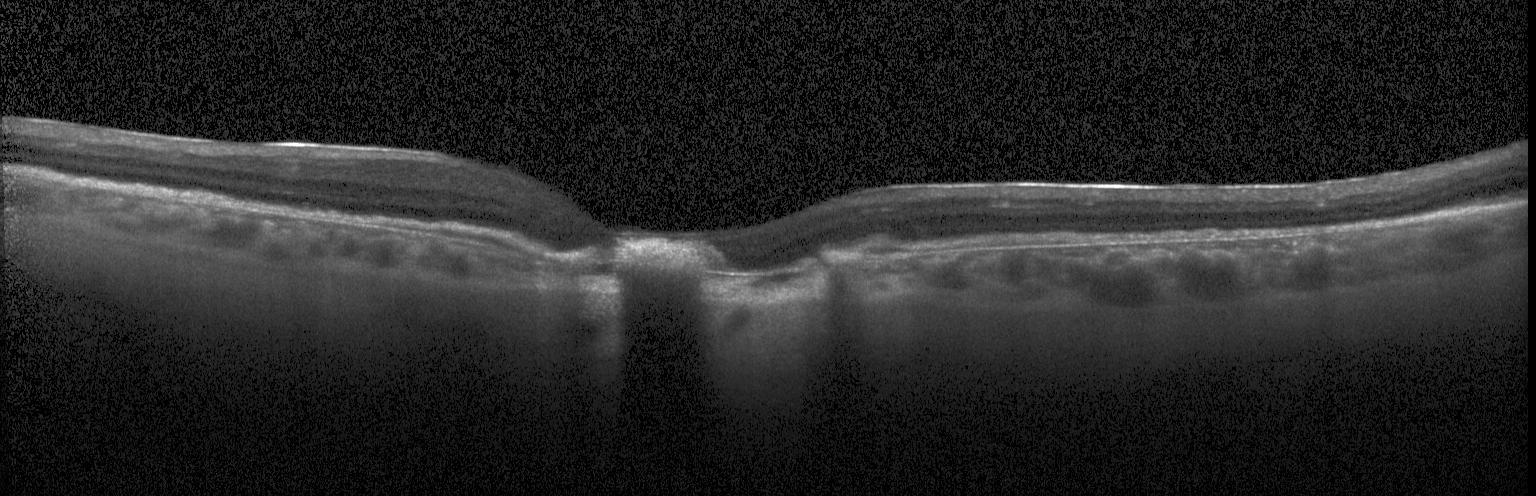
Spectral-domain OCT, OCT B-scan, instrument: Heidelberg Spectralis — A choroidal neovascular membrane.